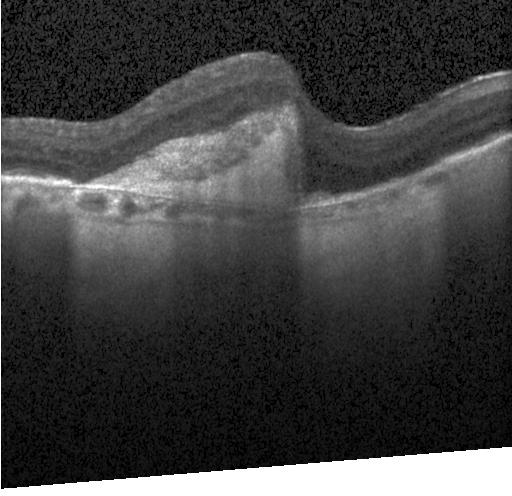

Spectral-domain optical coherence tomography; optical coherence tomography scan
Diagnosis: a choroidal neovascular membrane.